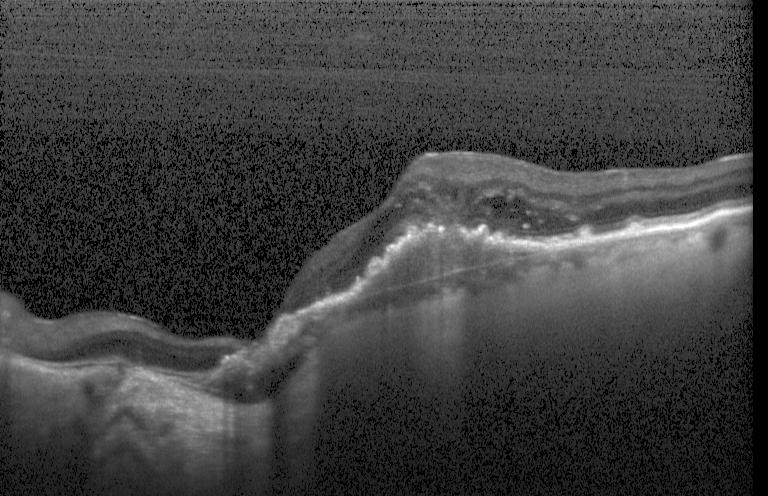

Diagnosis: a choroidal neovascular membrane.